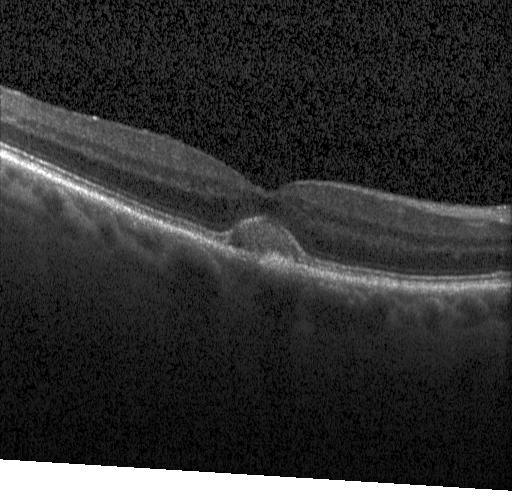
Retinal OCT B-scan; spectral-domain OCT; instrument: Heidelberg Spectralis — OCT finding: choroidal neovascularization (CNV).